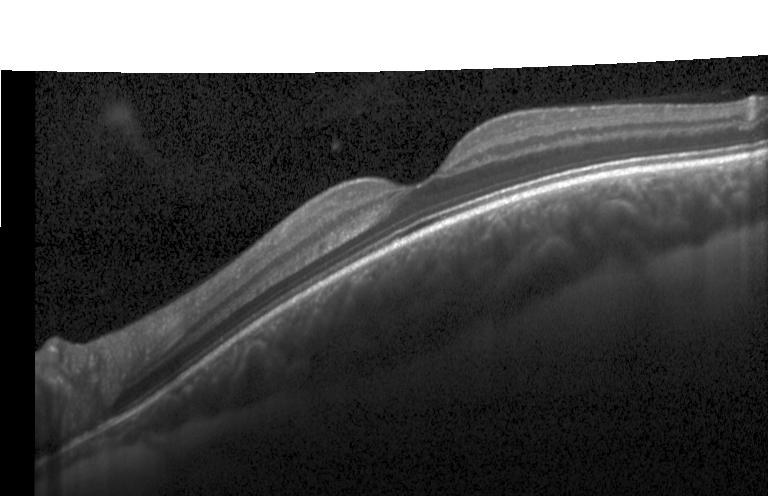
Spectral-domain OCT B-scan: no choroidal neovascularization, diabetic macular edema, or drusen.